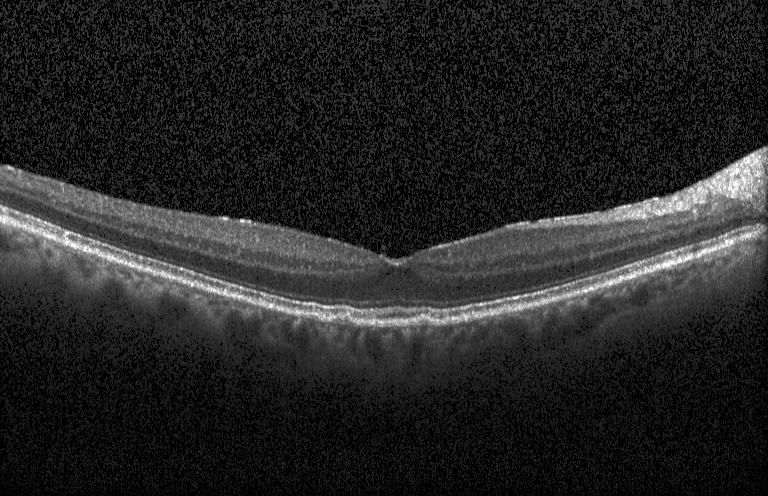

Spectral-domain OCT; optical coherence tomography B-scan; macular scan; Heidelberg Spectralis
Macular OCT: sub-RPE drusenoid deposits.